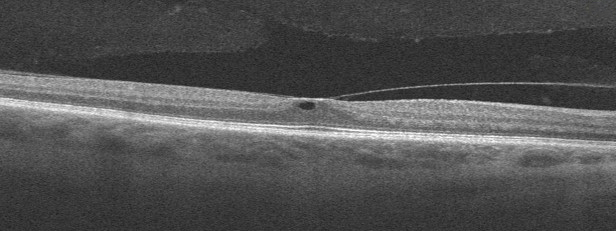 Retinal OCT B-scan — Assessment: vitreomacular interface disease (VID).